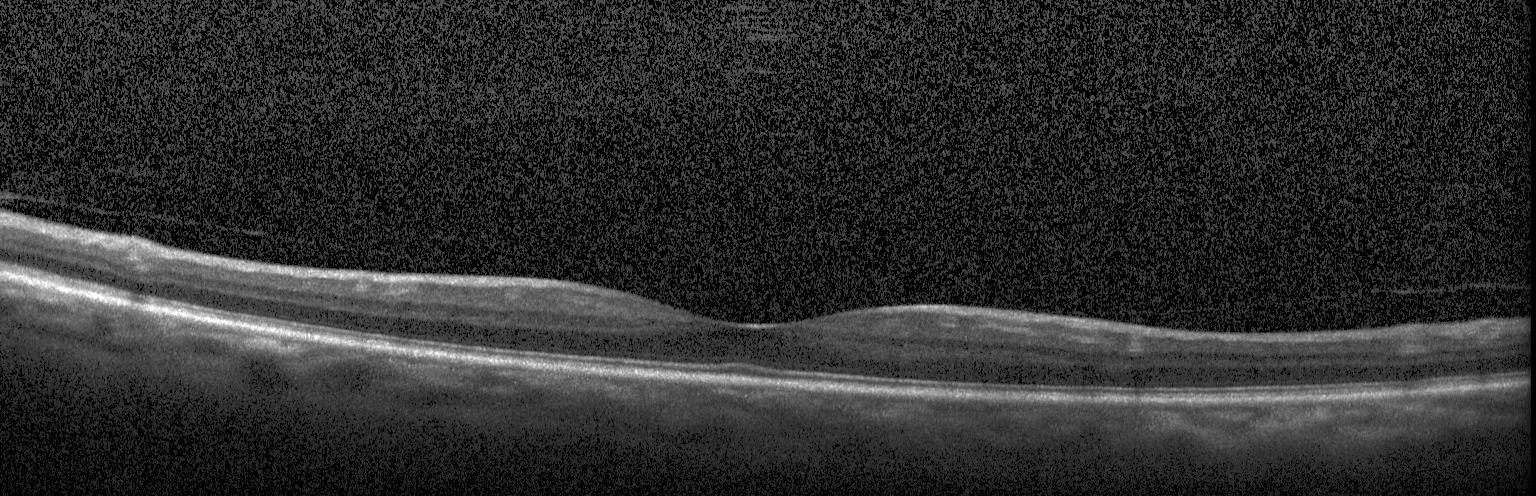
Spectral-domain OCT B-scan: no choroidal neovascularization, no diabetic macular edema, and no drusen.